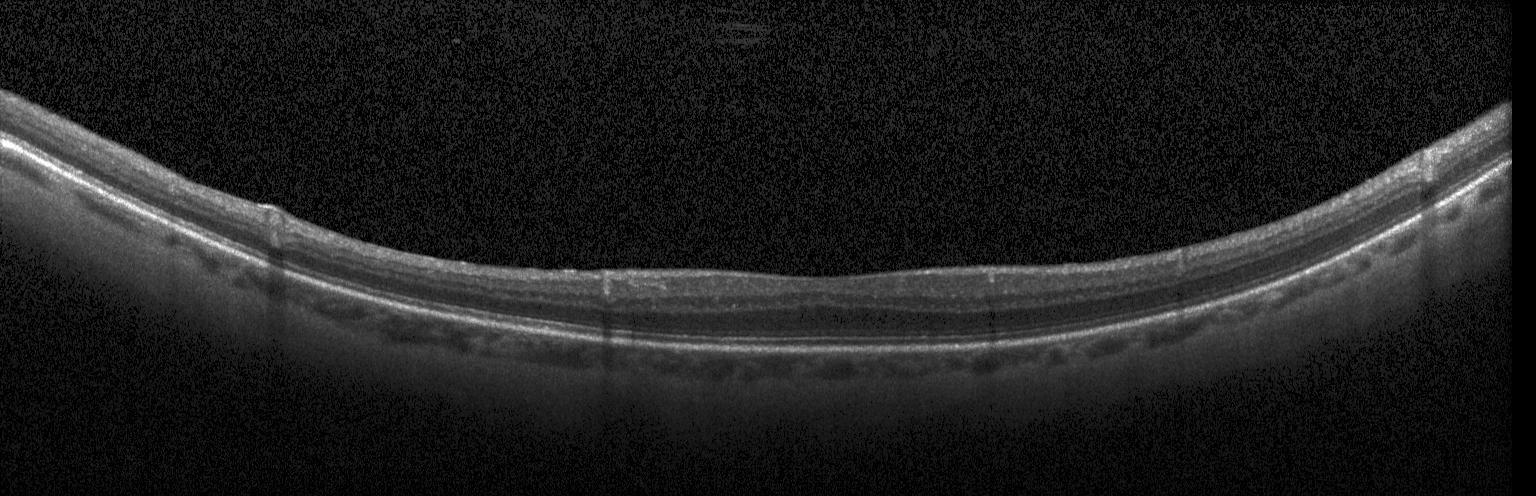

Finding: no CNV, DME, or drusen.